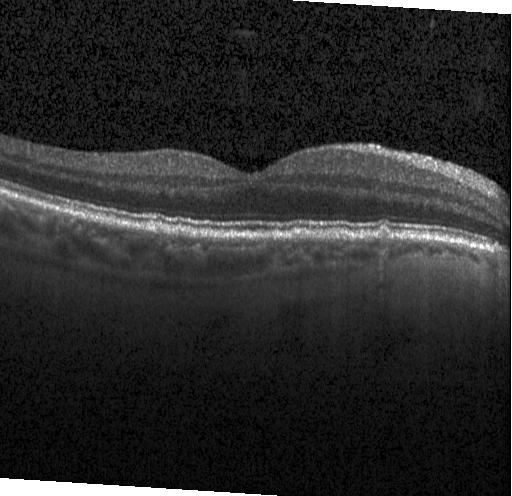 Assessment: sub-RPE drusenoid deposits.